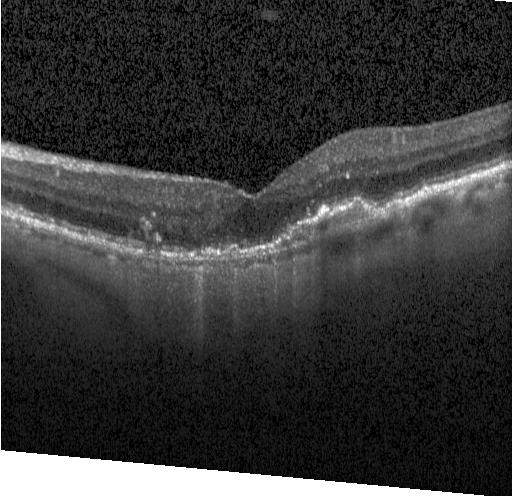
Heidelberg Spectralis OCT system; OCT line scan — Finding: a choroidal neovascular membrane.